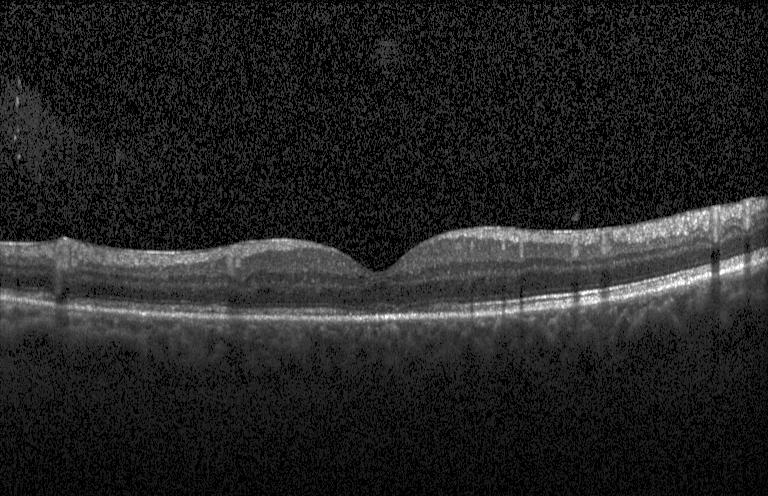

OCT B-scan; spectral-domain OCT; through the macula; Heidelberg Spectralis OCT system.
Neither choroidal neovascularization, diabetic macular edema, nor drusen.